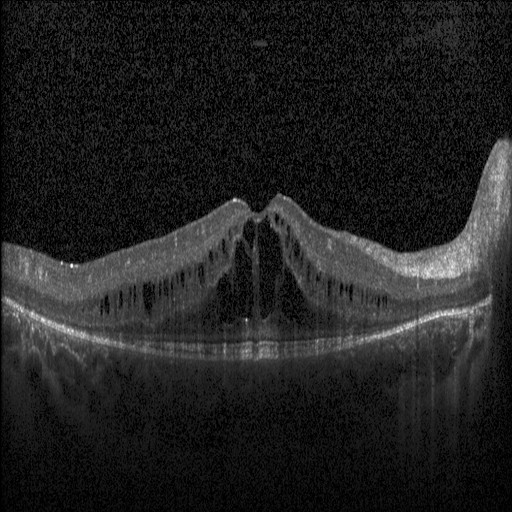 OCT finding: diabetic macular edema (DME).